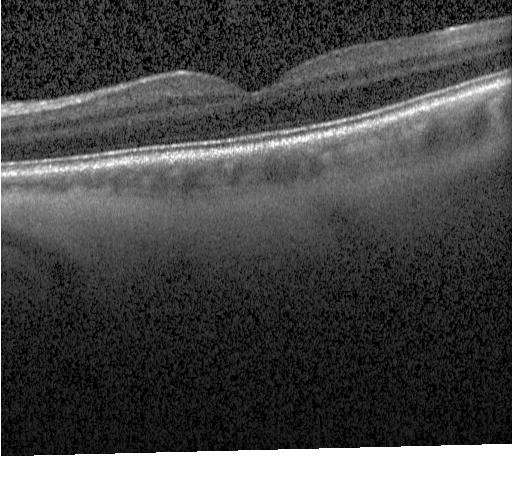 Macular OCT: no choroidal neovascularization, no diabetic macular edema, and no drusen.